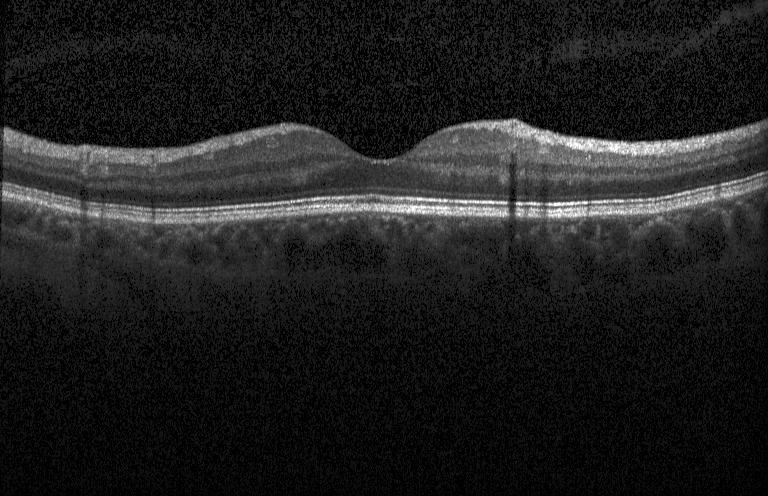
Spectral-domain OCT, Heidelberg Spectralis OCT system, optical coherence tomography B-scan, through the macula
No choroidal neovascularization, no diabetic macular edema, and no drusen.